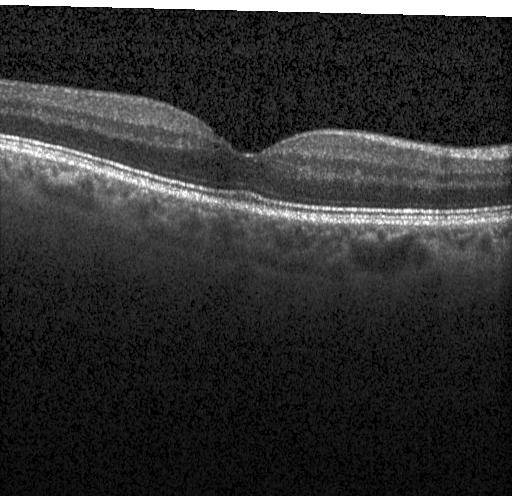
Retinal OCT cross-section showing no evidence of choroidal neovascularization, diabetic macular edema, or drusen.